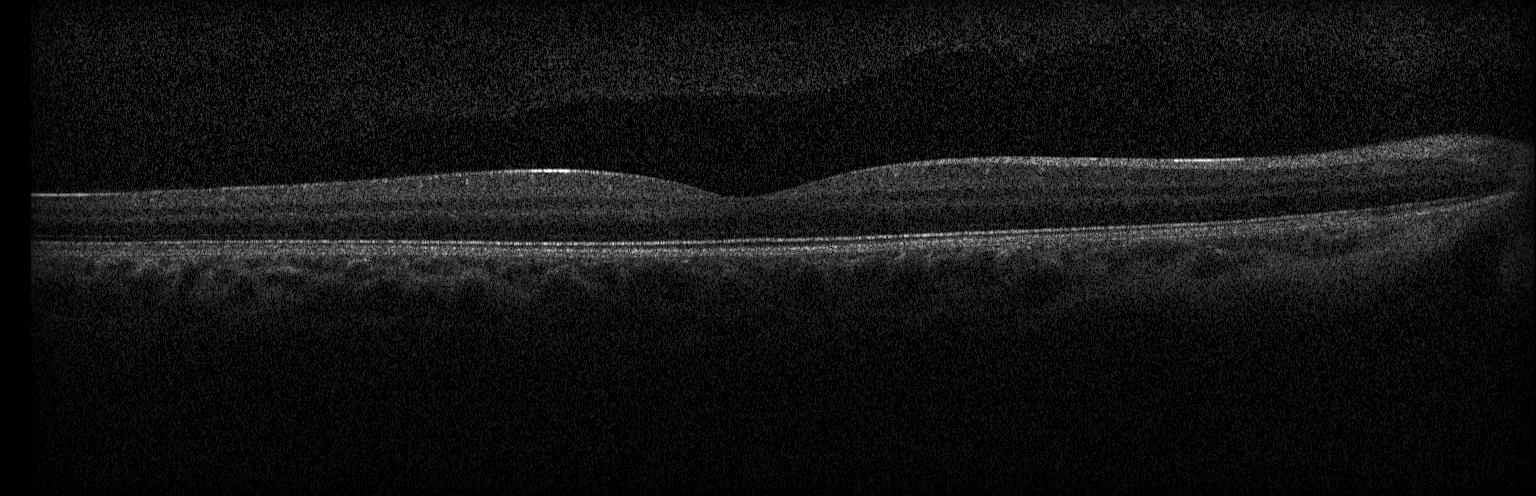
Diagnosis: no evidence of choroidal neovascularization, diabetic macular edema, or drusen.